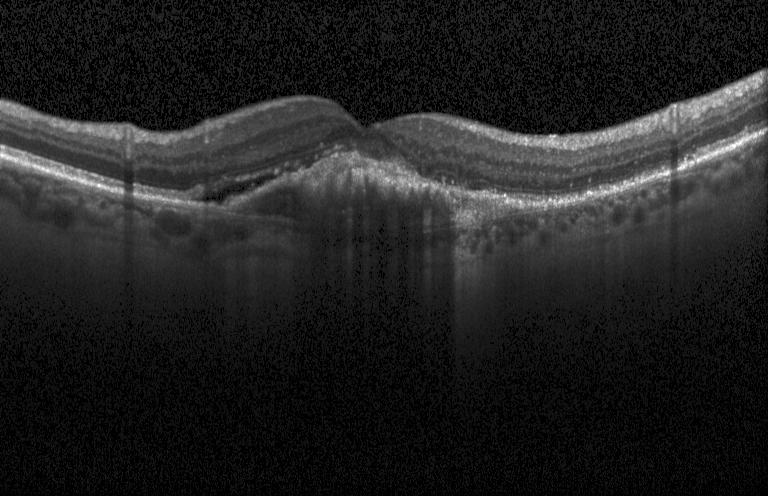
Heidelberg Spectralis · OCT line scan · spectral-domain optical coherence tomography · fovea-centered
Finding: a choroidal neovascular membrane.